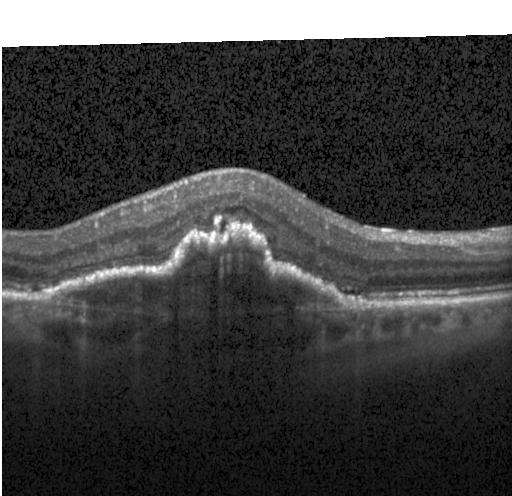 Spectral-domain OCT B-scan: a choroidal neovascular membrane.